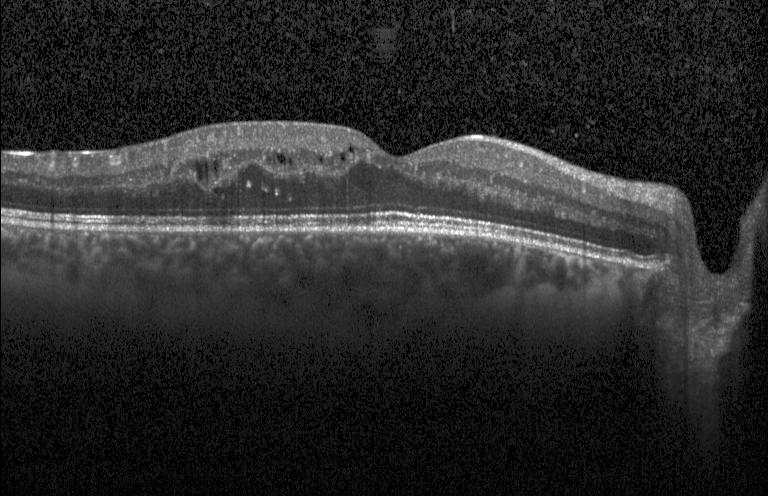
OCT line scan
Dx: diabetic macular edema (DME).